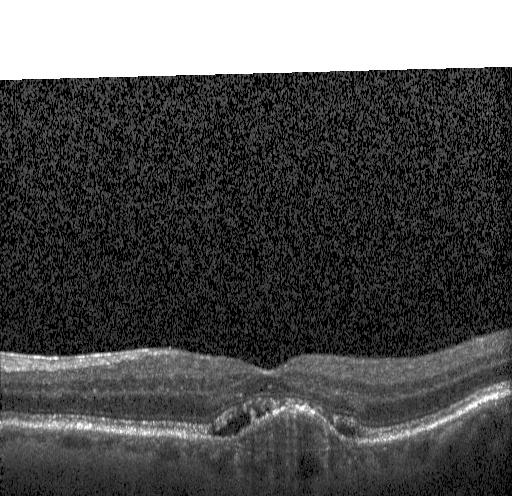 OCT B-scan.
Macular OCT: a choroidal neovascular membrane.